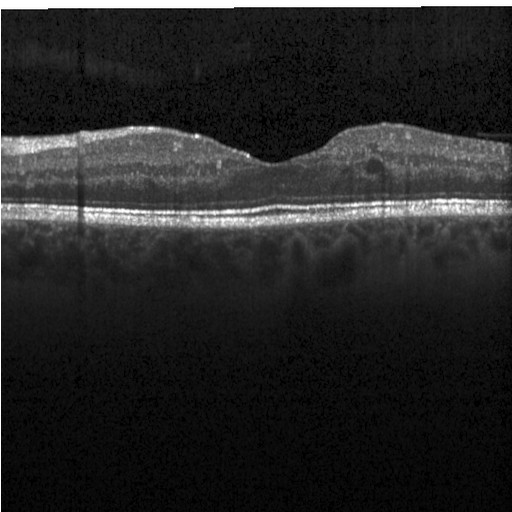

Fovea-centered. OCT B-scan. Heidelberg Spectralis OCT system. Finding: diabetic macular edema.